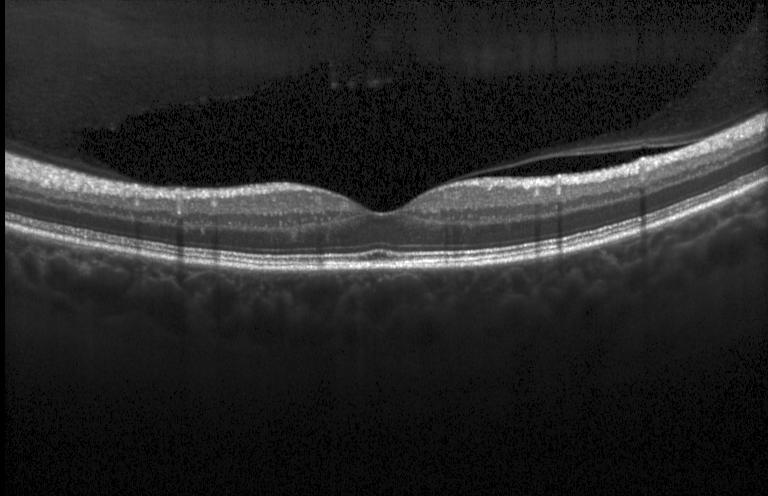 OCT line scan · SD-OCT.
The scan shows no choroidal neovascularization, no diabetic macular edema, and no drusen.